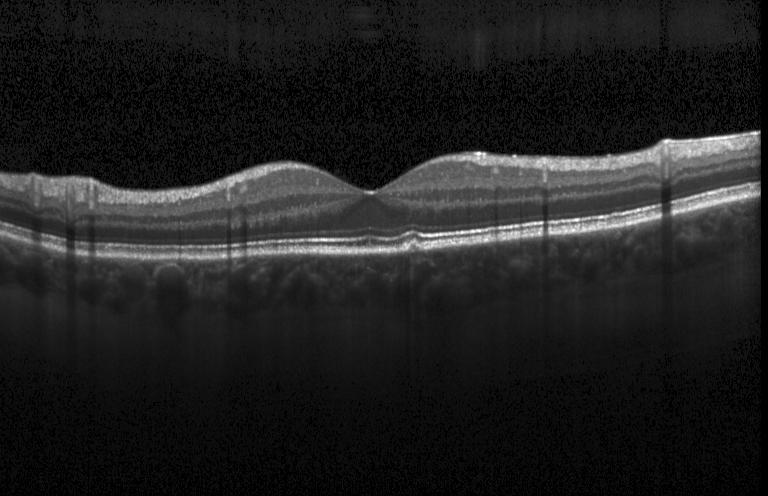

This B-scan demonstrates multiple drusen.